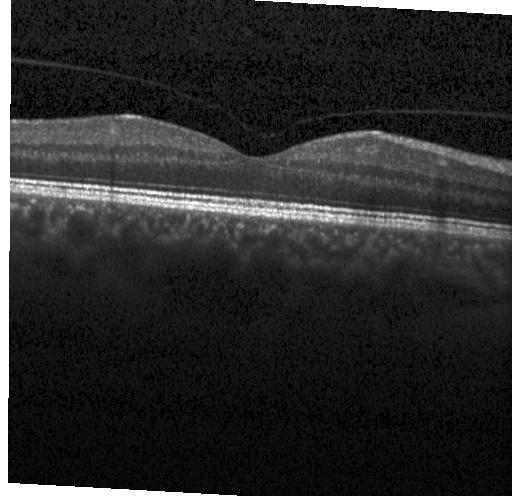
OCT line scan.
Diagnosis: no evidence of CNV, DME, or drusen.